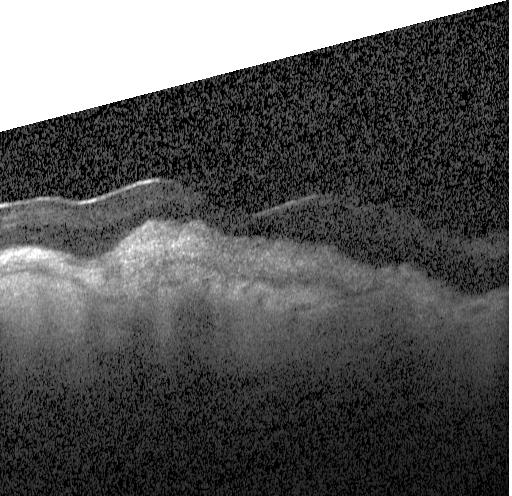

OCT finding: a choroidal neovascular membrane.